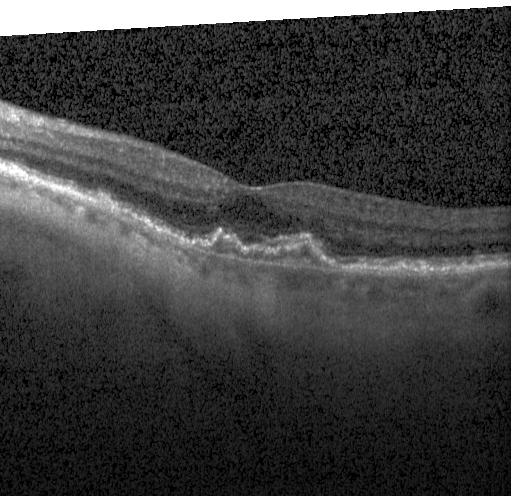
This B-scan demonstrates CNV.